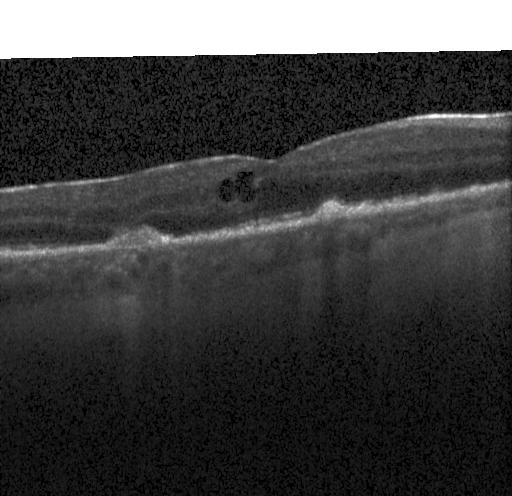 OCT line scan — Macular OCT: choroidal neovascularization (CNV).